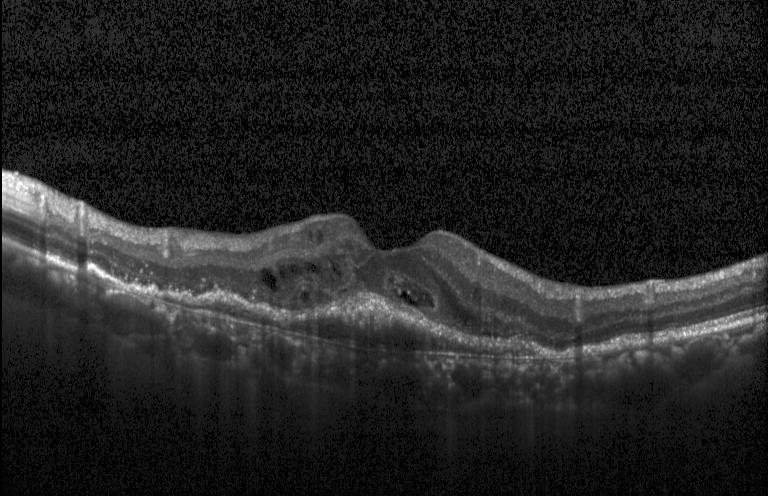

Finding: a choroidal neovascular membrane.